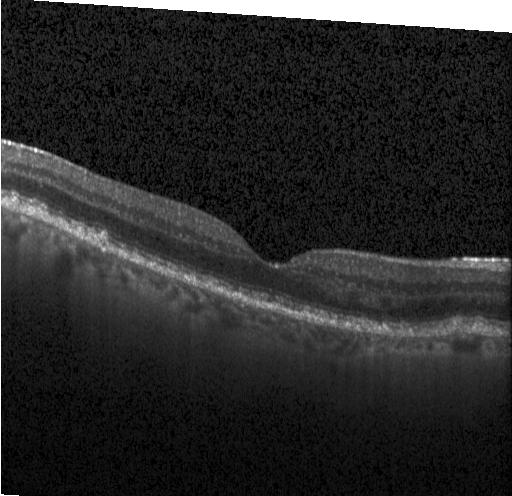
Diagnosis: drusen.